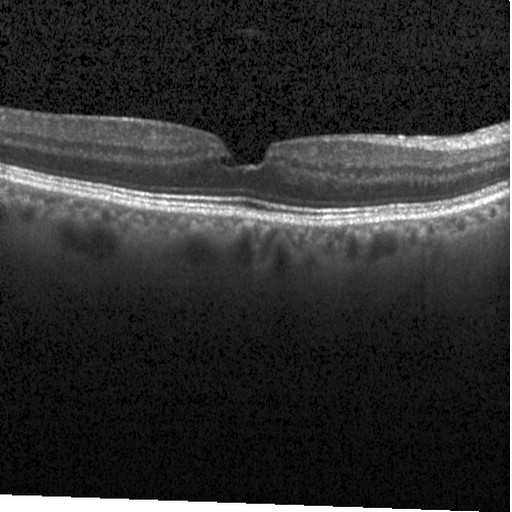 Through the macula, retinal OCT B-scan, spectral-domain optical coherence tomography — Diagnosis: diabetic macular edema.